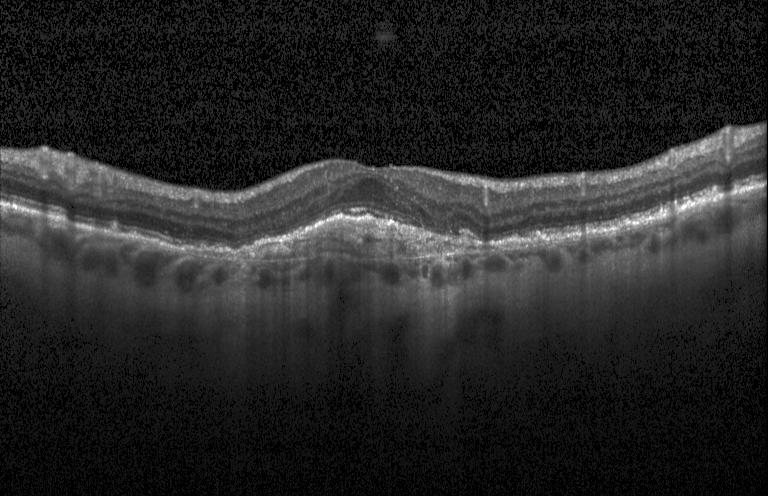

OCT line scan, acquired on a Heidelberg Spectralis. OCT finding: a choroidal neovascular membrane.